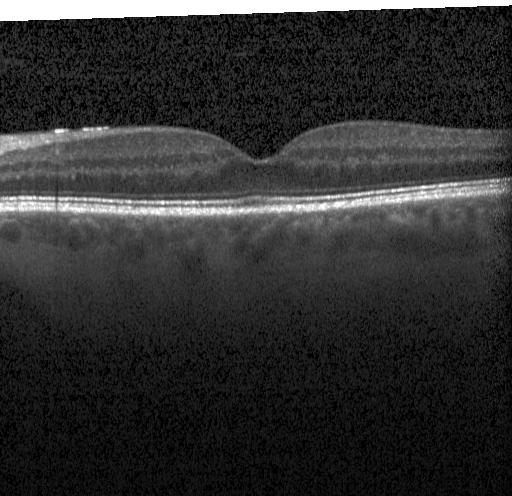

Diagnosis: no evidence of CNV, DME, or drusen.